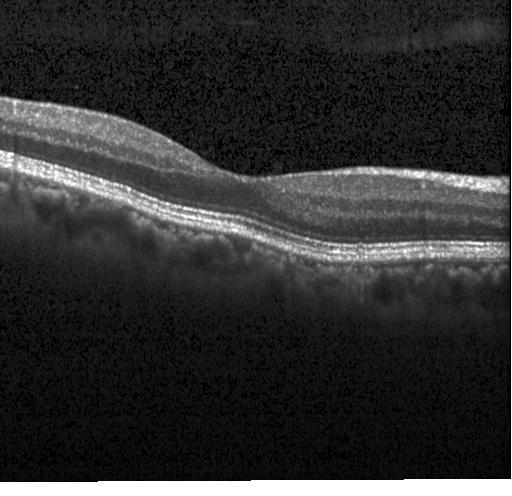 Optical coherence tomography B-scan. Dx: no evidence of CNV, DME, or drusen.